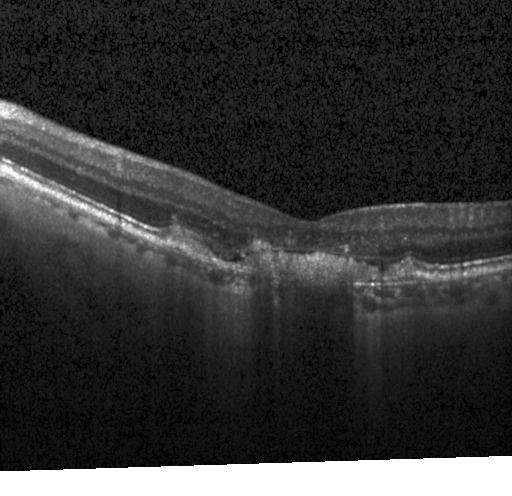
Finding: choroidal neovascularization (CNV).